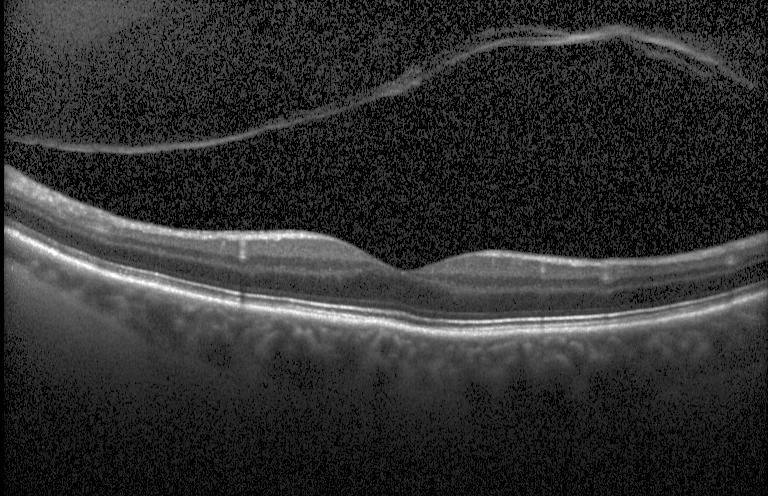
This B-scan demonstrates no evidence of choroidal neovascularization, diabetic macular edema, or drusen.